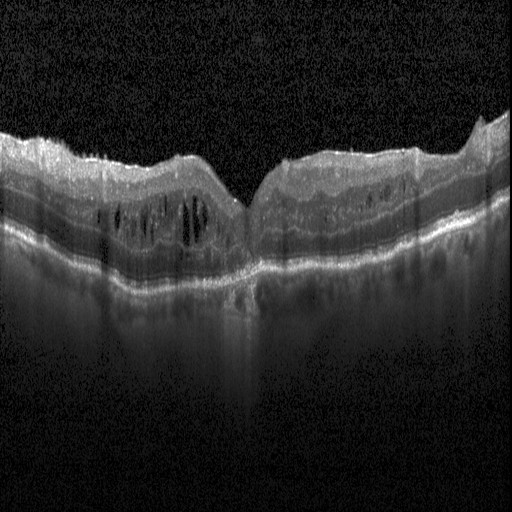
Retinal OCT B-scan; horizontal scan through the fovea; spectral-domain optical coherence tomography; instrument: Heidelberg Spectralis. OCT finding: diabetic macular edema.